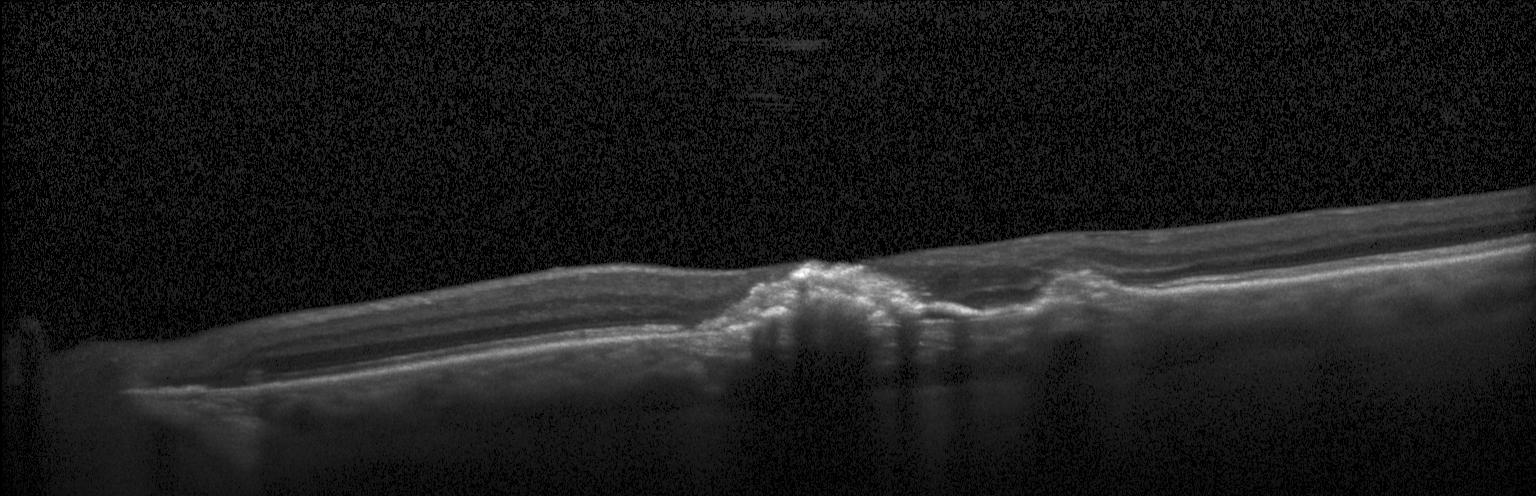 Retinal OCT B-scan.
Diagnosis: a choroidal neovascular membrane.